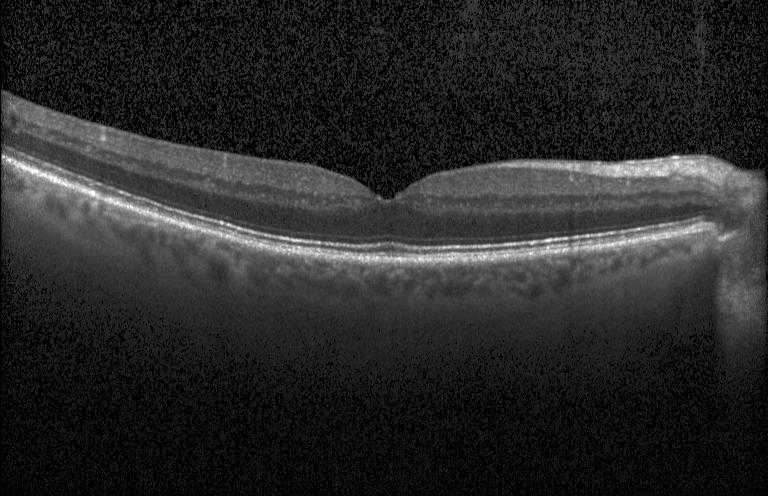 The scan shows no choroidal neovascularization, diabetic macular edema, or drusen.